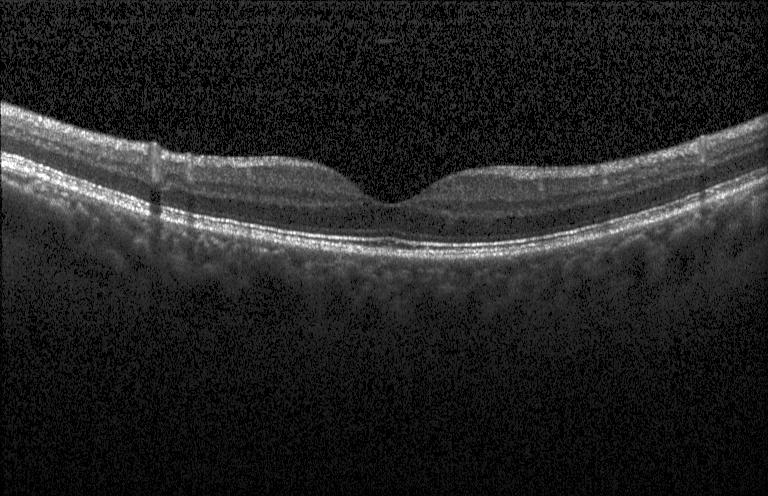
OCT B-scan showing neither choroidal neovascularization, diabetic macular edema, nor drusen.